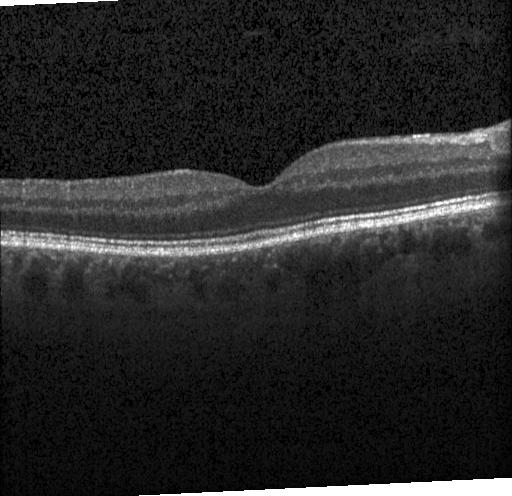

Macular OCT: no choroidal neovascularization, diabetic macular edema, or drusen.